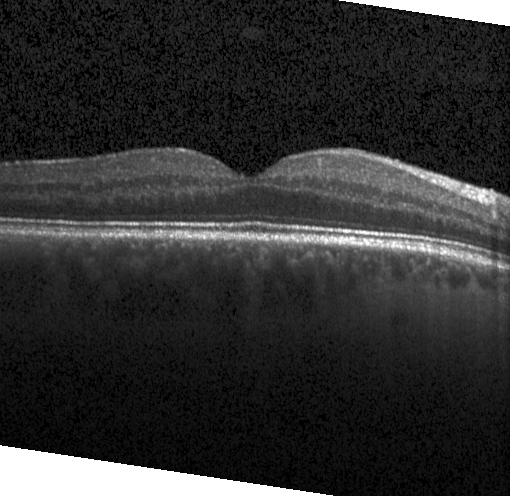
Heidelberg Spectralis. OCT line scan
Assessment: no choroidal neovascularization, diabetic macular edema, or drusen.